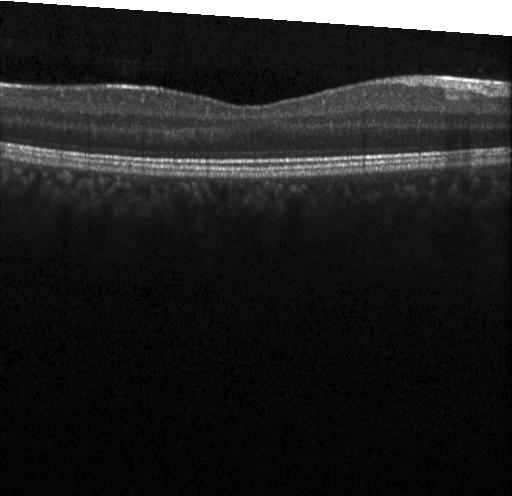

Acquired on a Heidelberg Spectralis, OCT B-scan, fovea-centered, spectral-domain OCT.
Diagnosis: no evidence of choroidal neovascularization, diabetic macular edema, or drusen.